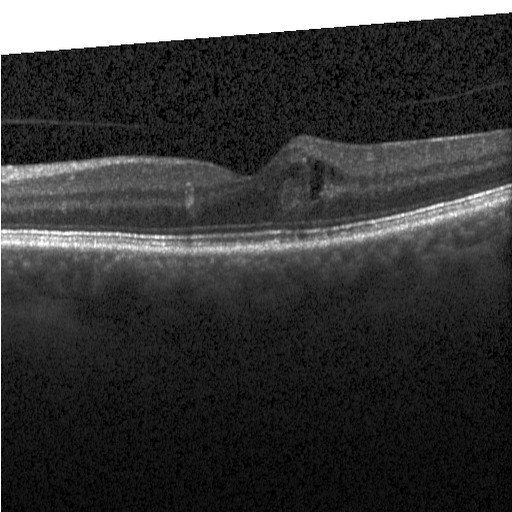

This B-scan demonstrates diabetic macular edema.